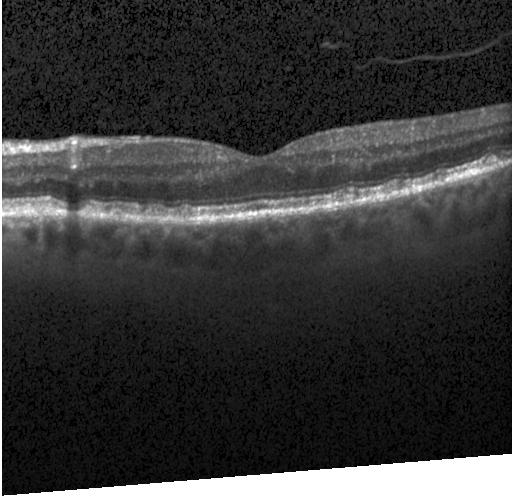
Centered on the fovea. Heidelberg Spectralis OCT system. Spectral-domain OCT. Retinal OCT B-scan.
This B-scan demonstrates multiple drusen.